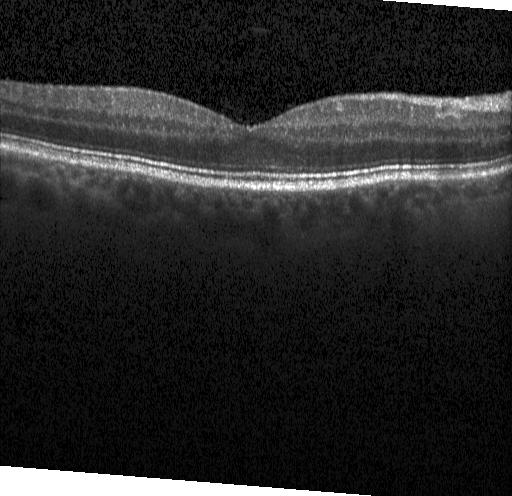
Instrument: Heidelberg Spectralis. Through the macula. Retinal OCT cross-section. Finding: neither CNV, DME, nor drusen.